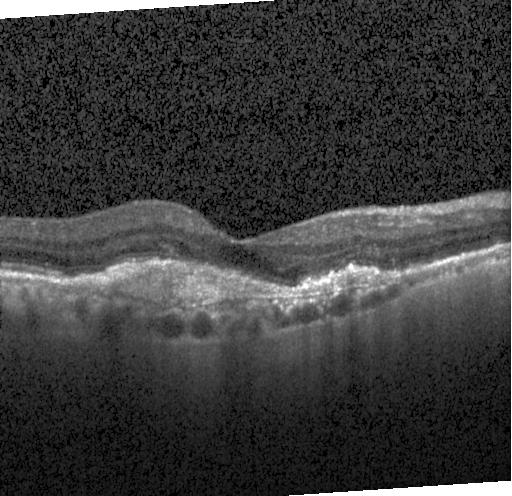

Heidelberg Spectralis OCT system, centered on the fovea, OCT B-scan. This B-scan demonstrates a choroidal neovascular membrane.